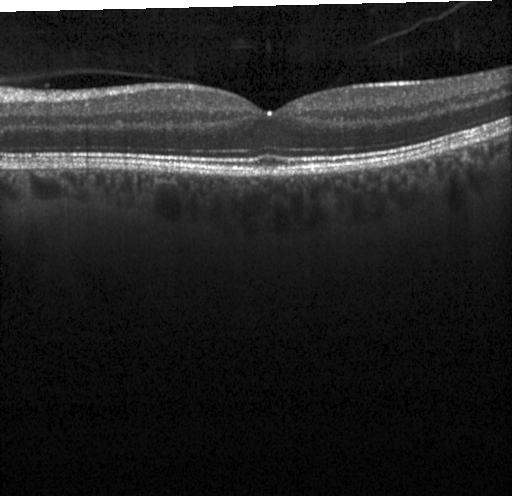 Heidelberg Spectralis. Through the macula. Spectral-domain optical coherence tomography. Optical coherence tomography B-scan — No evidence of choroidal neovascularization, diabetic macular edema, or drusen.